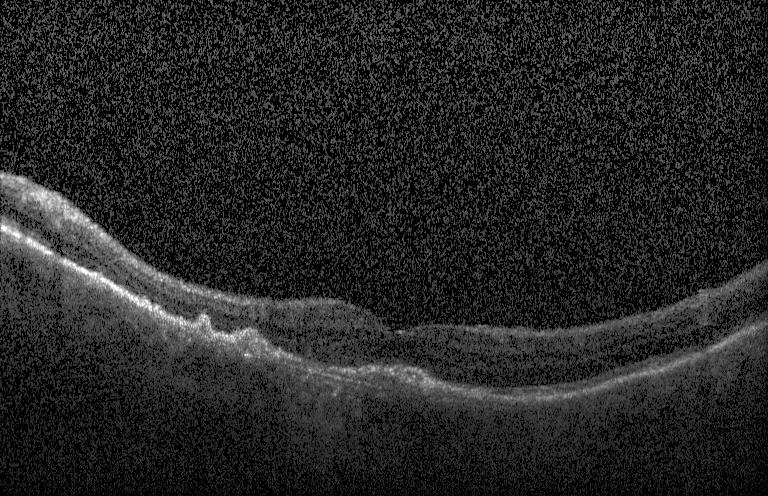

OCT finding: choroidal neovascularization.